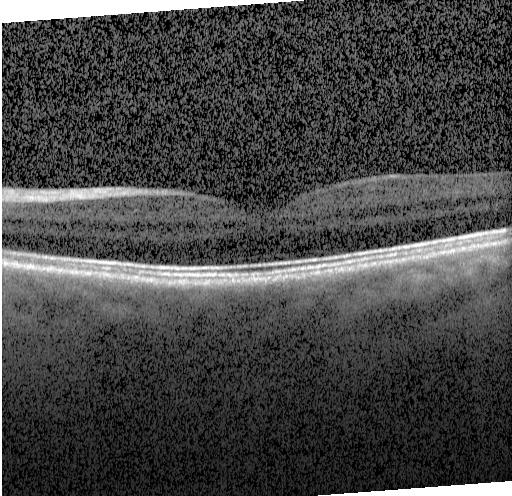 Spectral-domain optical coherence tomography · through the macula · instrument: Heidelberg Spectralis · optical coherence tomography scan. Assessment: no choroidal neovascularization, no diabetic macular edema, and no drusen.